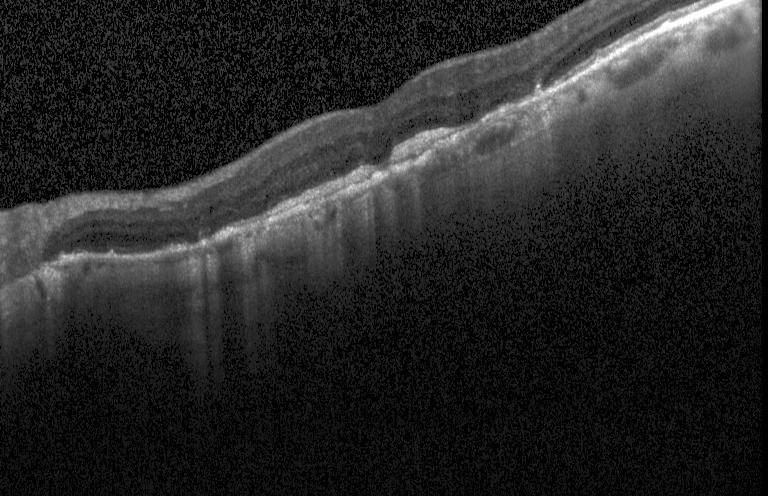 Acquired on a Heidelberg Spectralis · SD-OCT · optical coherence tomography B-scan · horizontal scan through the fovea
Impression: choroidal neovascularization.